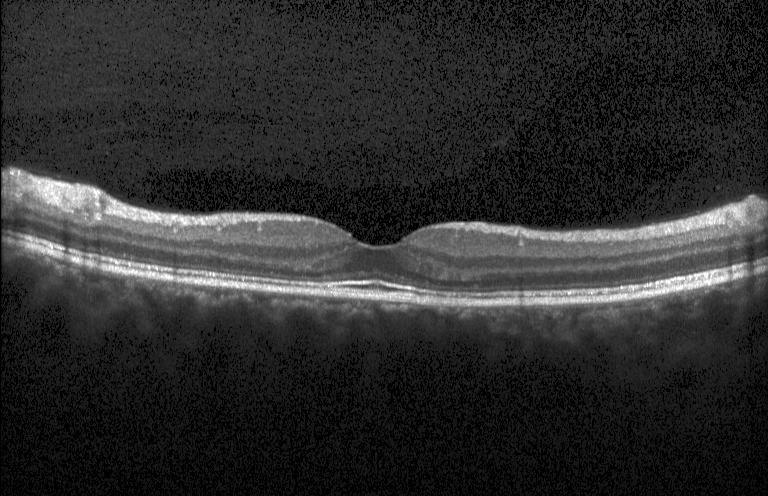

Optical coherence tomography scan
Impression: no choroidal neovascularization, diabetic macular edema, or drusen.